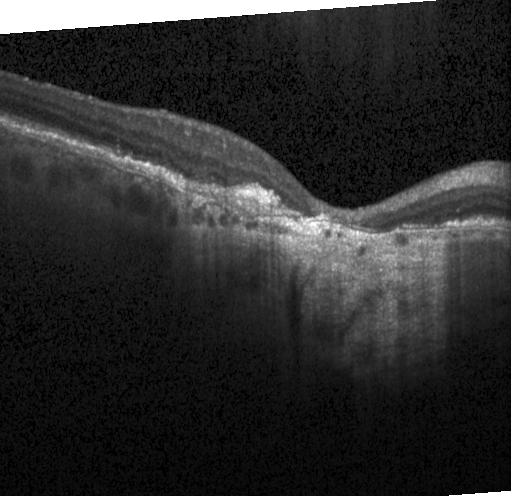

CNV.